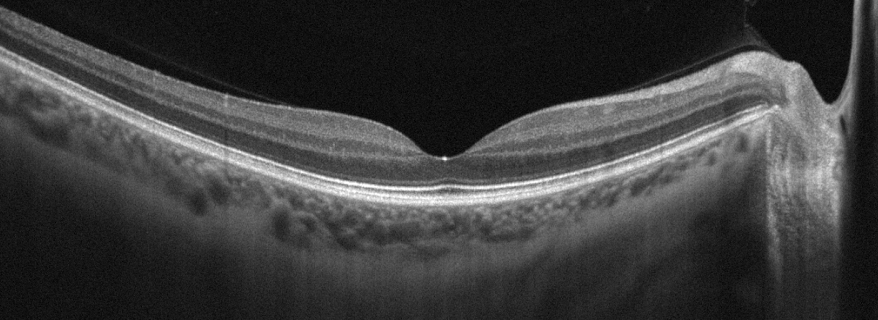

Retinal OCT B-scan.
Impression: no AMD, DME, ERM, RAO, RVO, or VID.